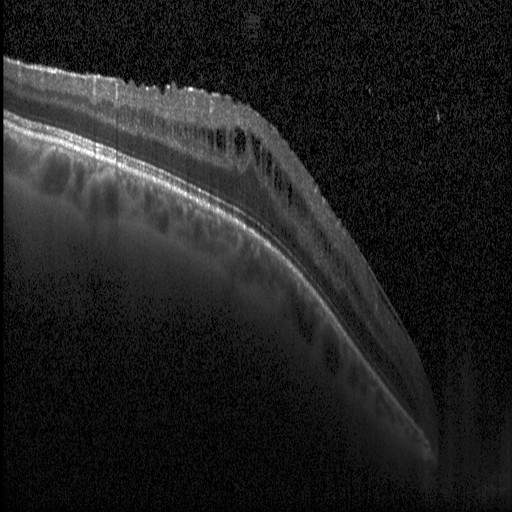 Through the macula. Optical coherence tomography B-scan.
OCT finding: diabetic macular edema (DME).